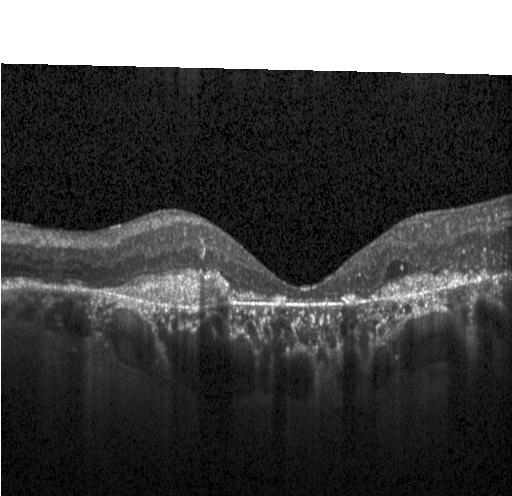
Heidelberg Spectralis OCT system; retinal OCT cross-section.
Diagnosis: CNV.